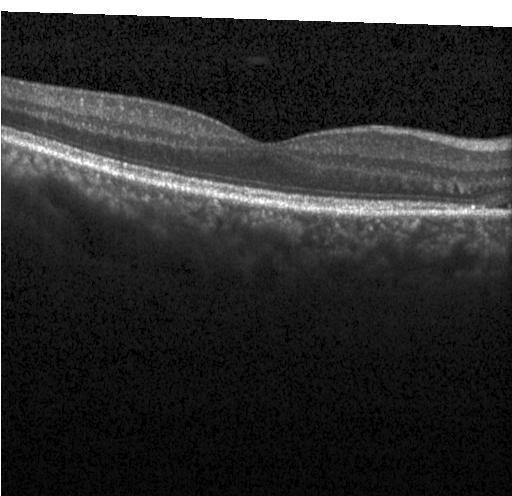
Fovea-centered. OCT line scan.
Finding: no choroidal neovascularization, diabetic macular edema, or drusen.